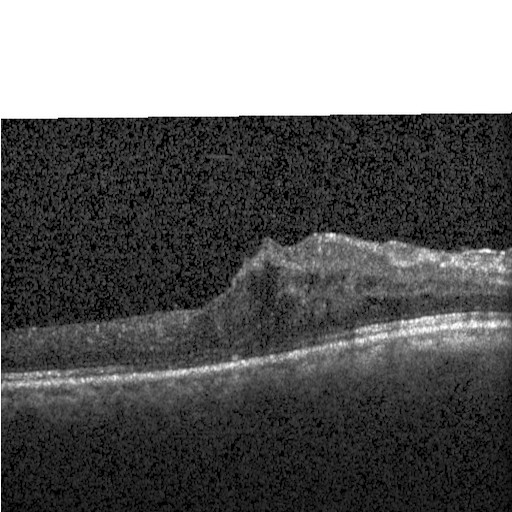
Spectral-domain OCT B-scan: diabetic macular edema (DME).